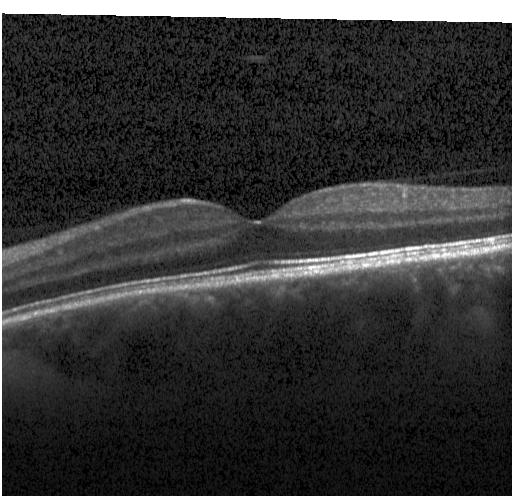

OCT B-scan.
Finding: no choroidal neovascularization, diabetic macular edema, or drusen.